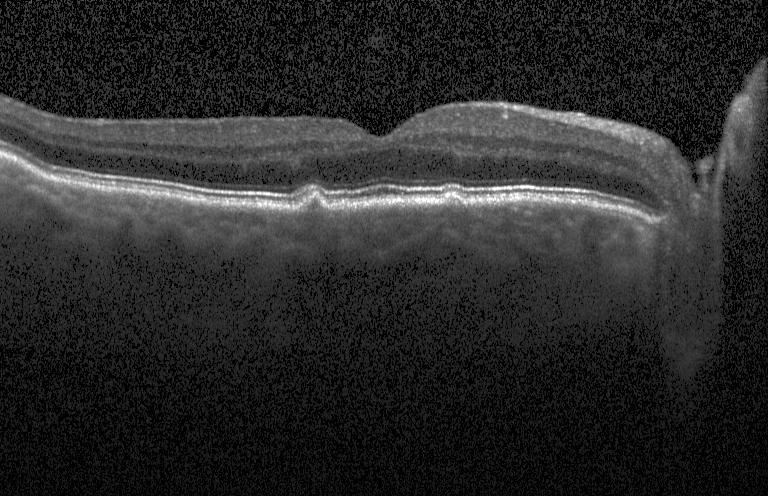
Optical coherence tomography B-scan, Heidelberg Spectralis — The scan shows drusen.